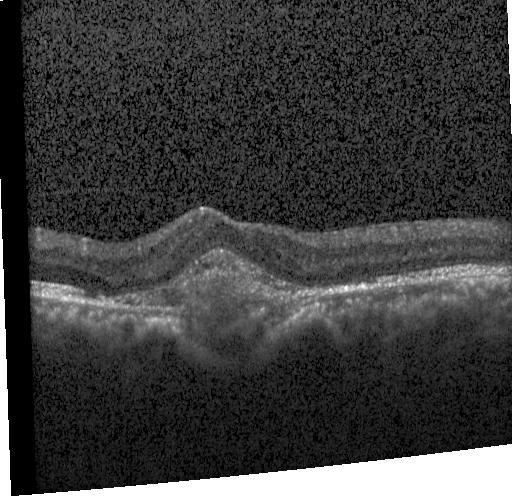
Horizontal scan through the fovea; SD-OCT; OCT B-scan; acquired on a Heidelberg Spectralis
Diagnosis: a choroidal neovascular membrane.